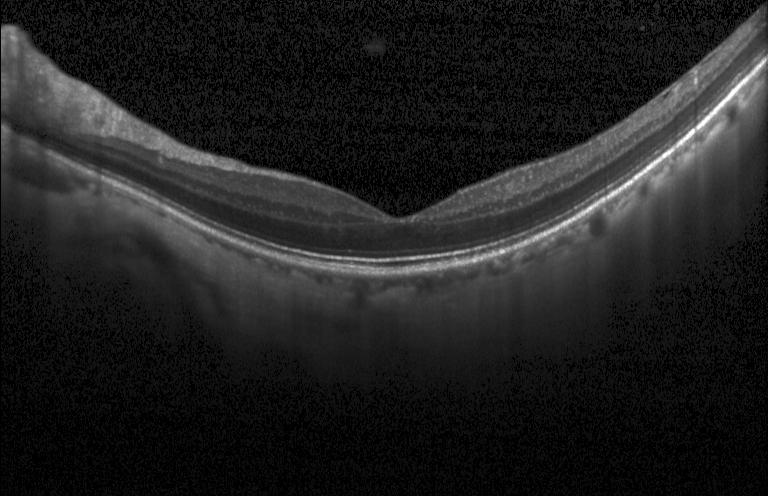 Neither CNV, DME, nor drusen.